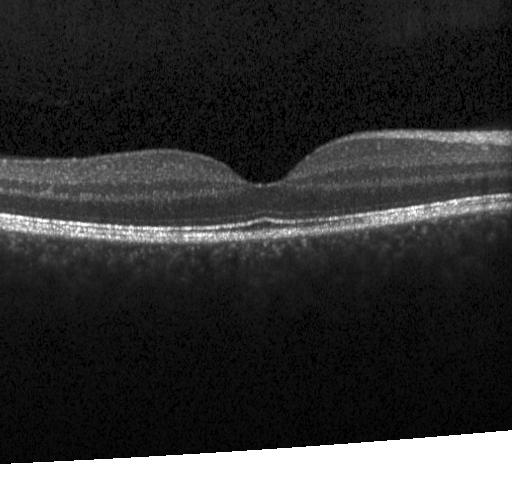
Finding: neither choroidal neovascularization, diabetic macular edema, nor drusen.